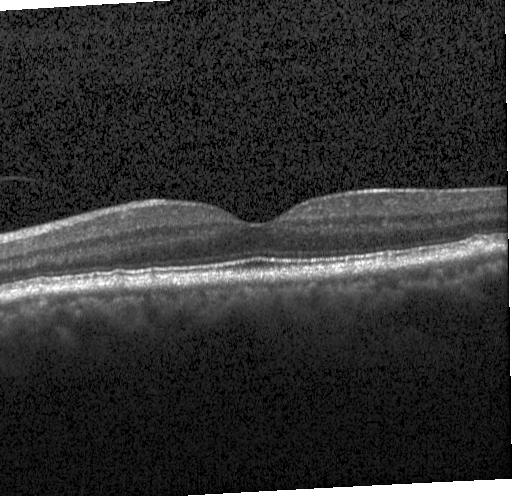 Optical coherence tomography scan.
Diagnosis: no evidence of CNV, DME, or drusen.